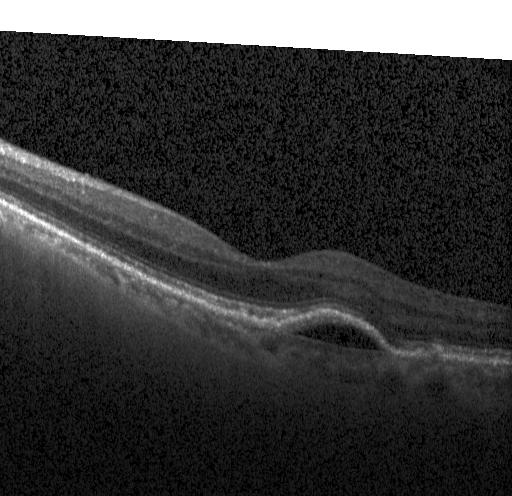
Retinal OCT cross-section showing choroidal neovascularization.